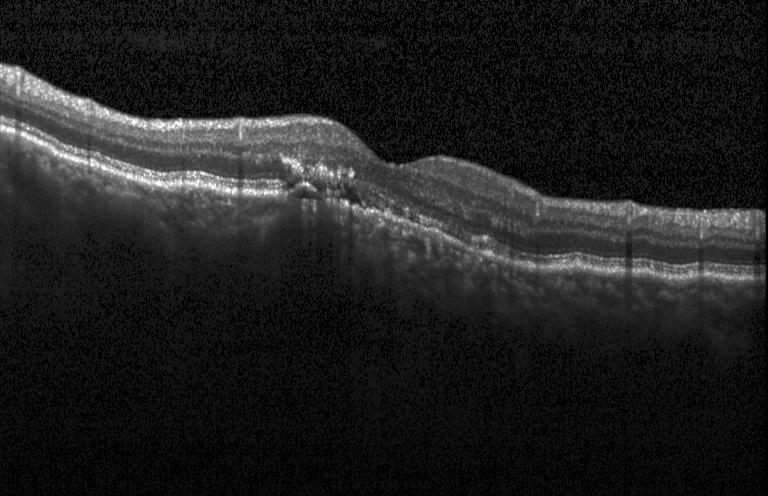

Heidelberg Spectralis OCT system; optical coherence tomography B-scan
The scan shows a choroidal neovascular membrane.